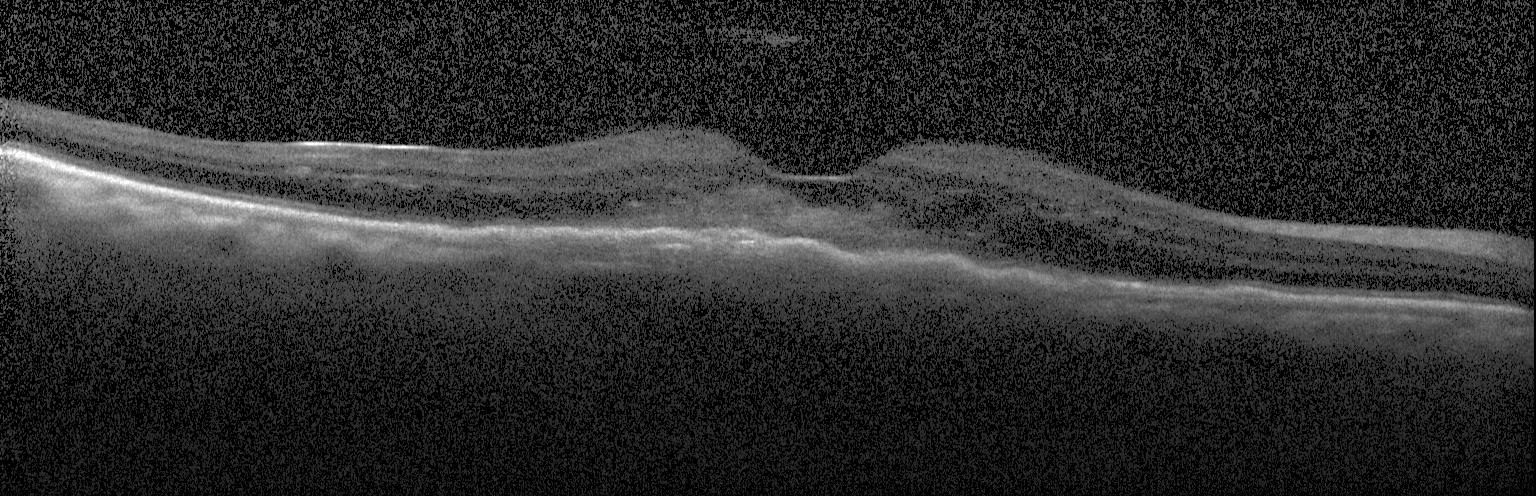 OCT scan showing a choroidal neovascular membrane.